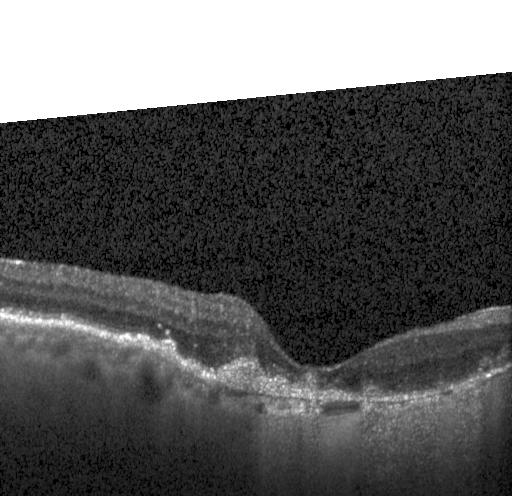
Diagnosis: a choroidal neovascular membrane.